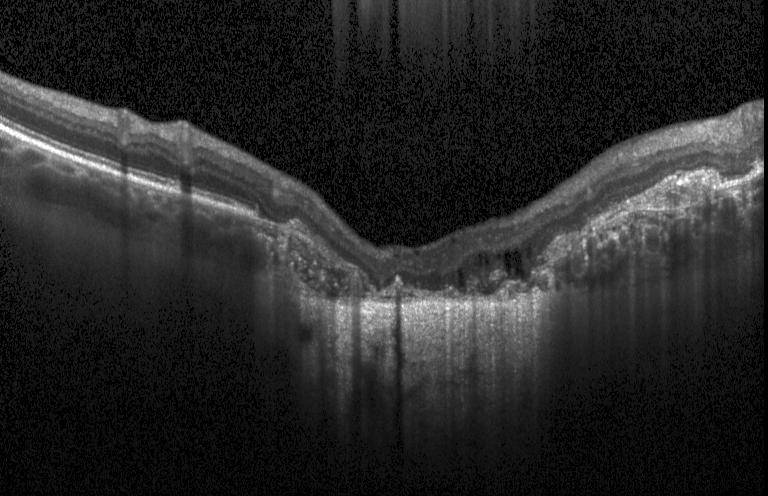

Optical coherence tomography scan — The scan shows a choroidal neovascular membrane.